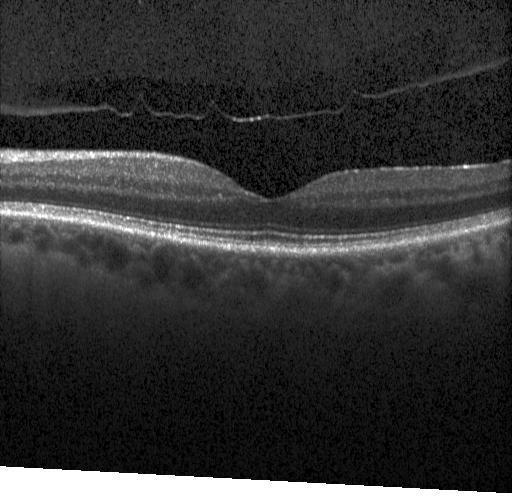

Spectral-domain OCT · fovea-centered · retinal OCT cross-section
No choroidal neovascularization, diabetic macular edema, or drusen.